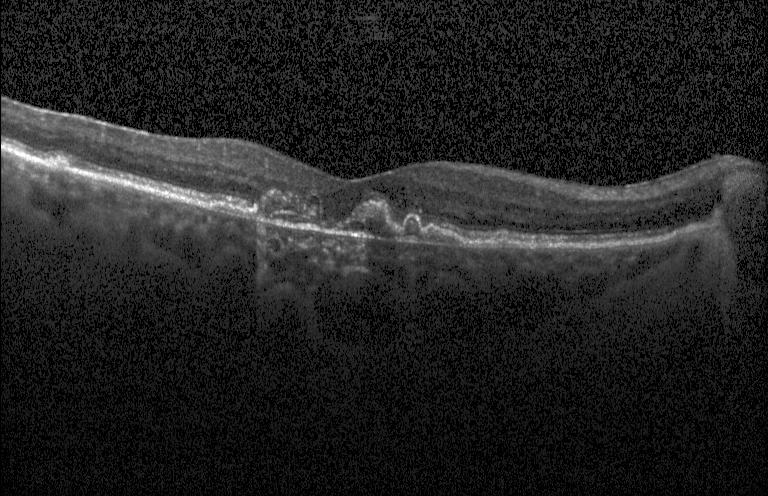

Instrument: Heidelberg Spectralis. Optical coherence tomography scan. Spectral-domain optical coherence tomography. Horizontal scan through the fovea — Macular OCT: choroidal neovascularization (CNV).